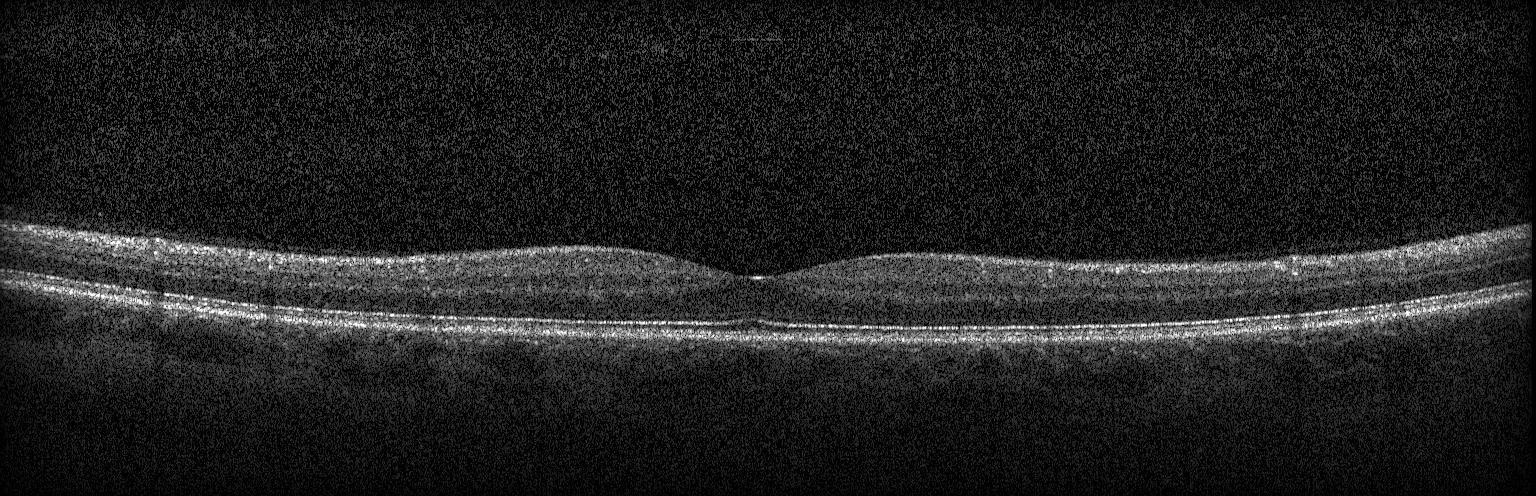
Finding: no choroidal neovascularization, diabetic macular edema, or drusen.